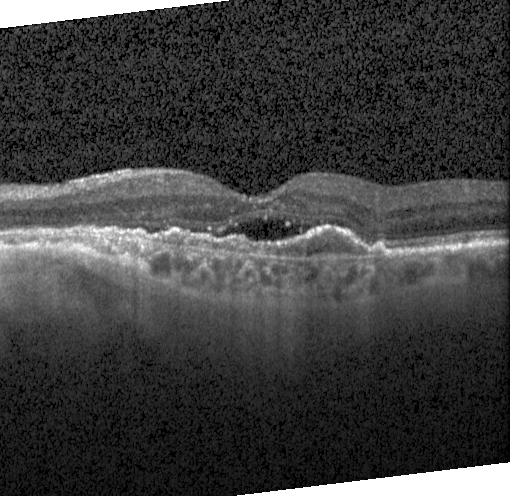 Macular OCT: CNV.